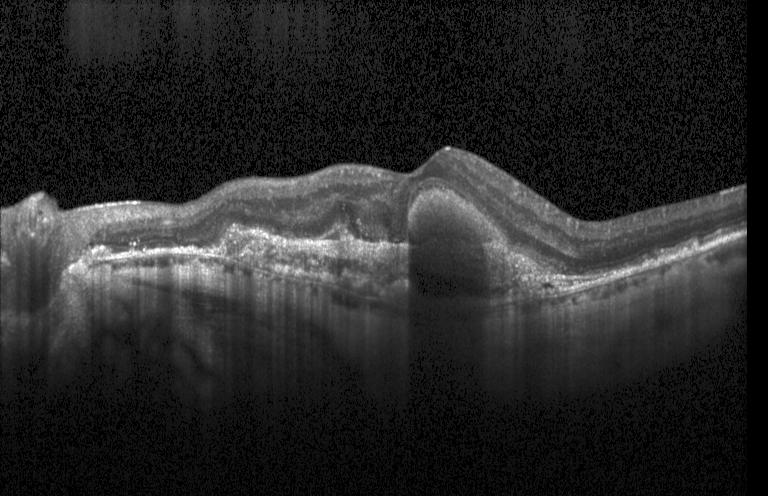

OCT finding: a choroidal neovascular membrane.